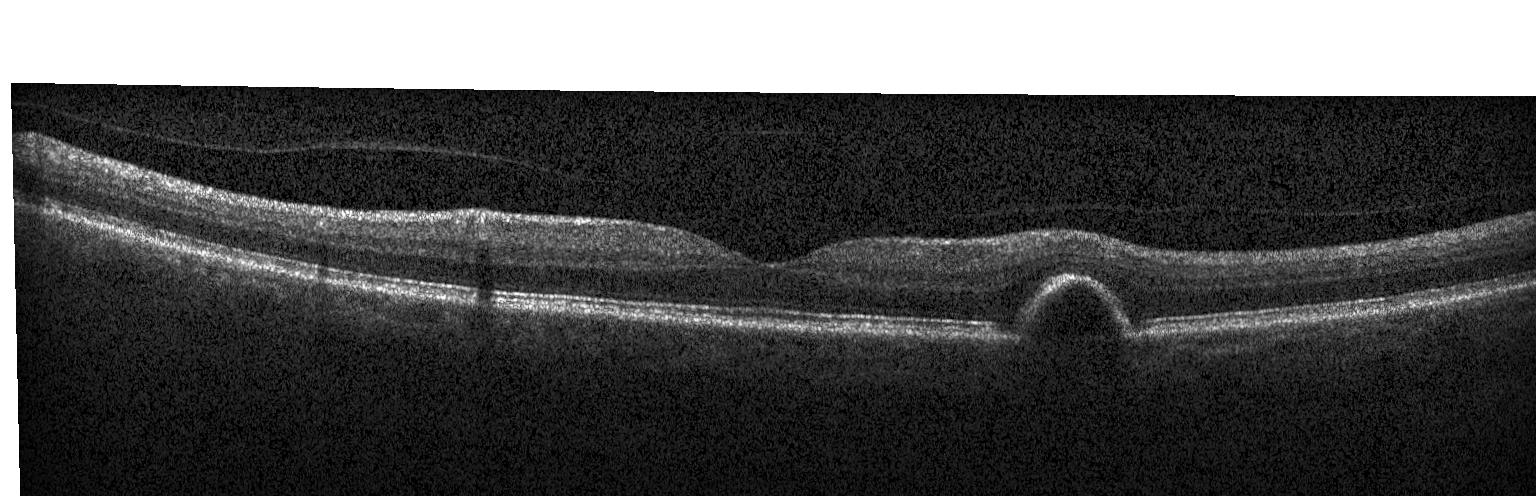 Macular scan, SD-OCT, OCT line scan
OCT finding: a choroidal neovascular membrane.